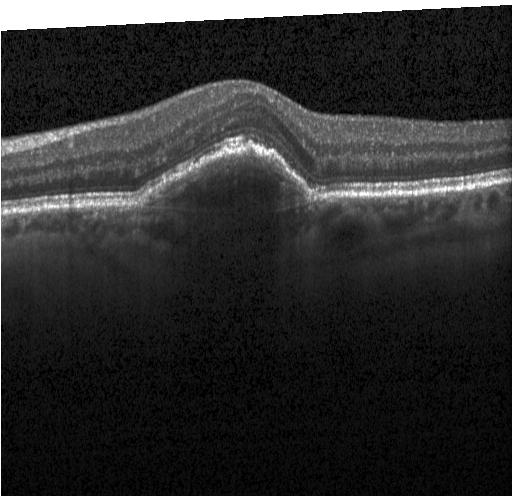 Diagnosis: a choroidal neovascular membrane.